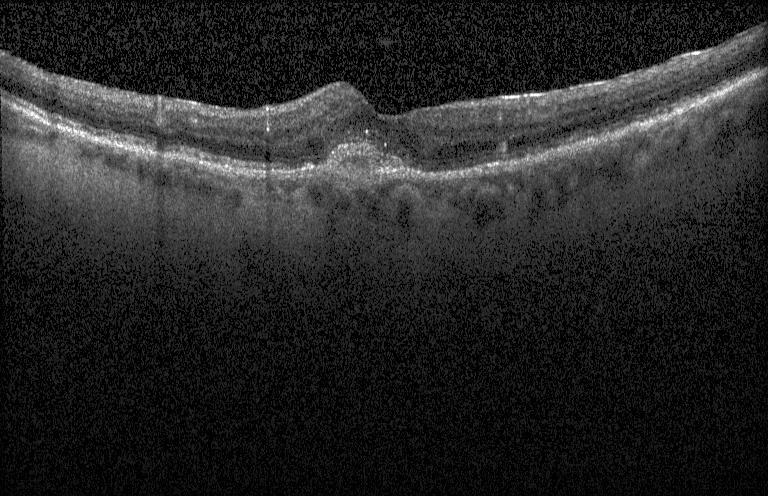 OCT finding: choroidal neovascularization.